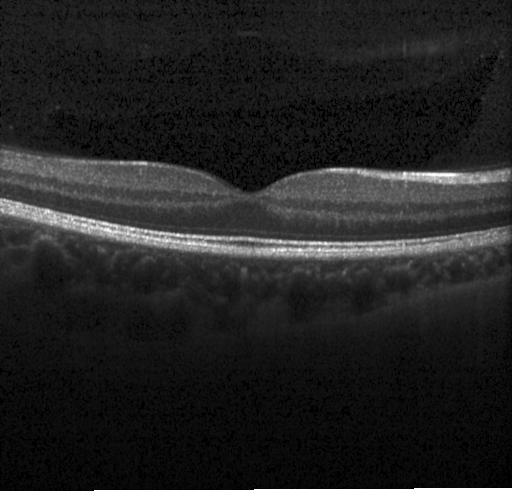
Retinal OCT cross-section. Diagnosis: no evidence of choroidal neovascularization, diabetic macular edema, or drusen.